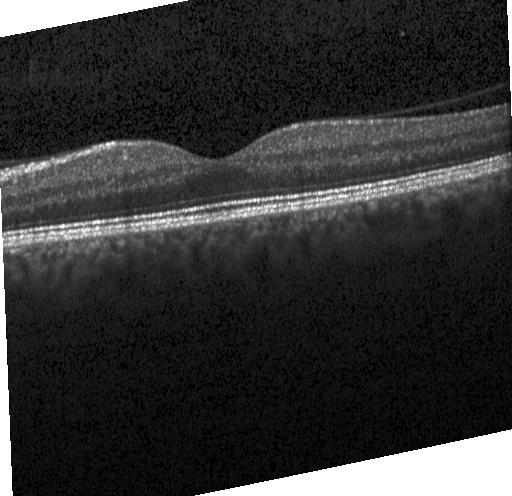 Instrument: Heidelberg Spectralis. Spectral-domain OCT. Retinal OCT B-scan — Finding: neither CNV, DME, nor drusen.